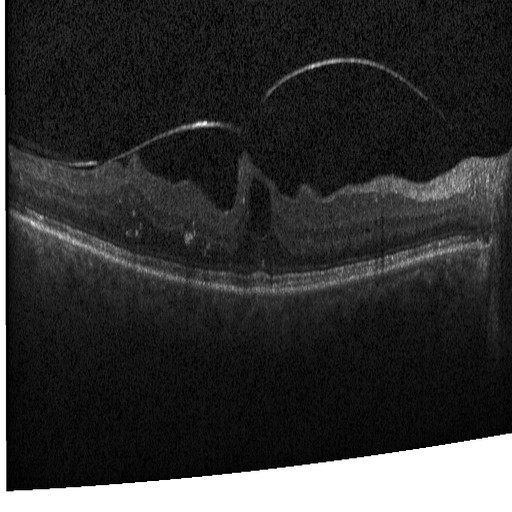

Spectral-domain optical coherence tomography, acquired on a Heidelberg Spectralis, optical coherence tomography scan, macular scan
Diagnosis: diabetic macular edema.